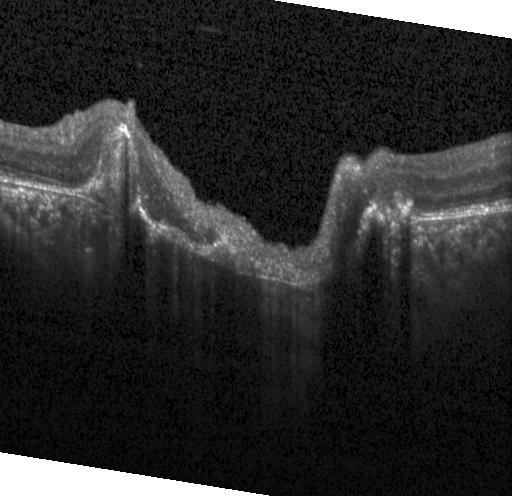
The scan shows a choroidal neovascular membrane.